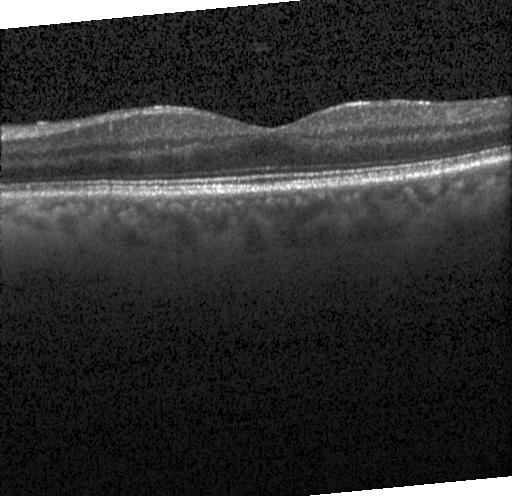

Fovea-centered · spectral-domain optical coherence tomography · acquired on a Heidelberg Spectralis · optical coherence tomography B-scan. Dx: no choroidal neovascularization, no diabetic macular edema, and no drusen.